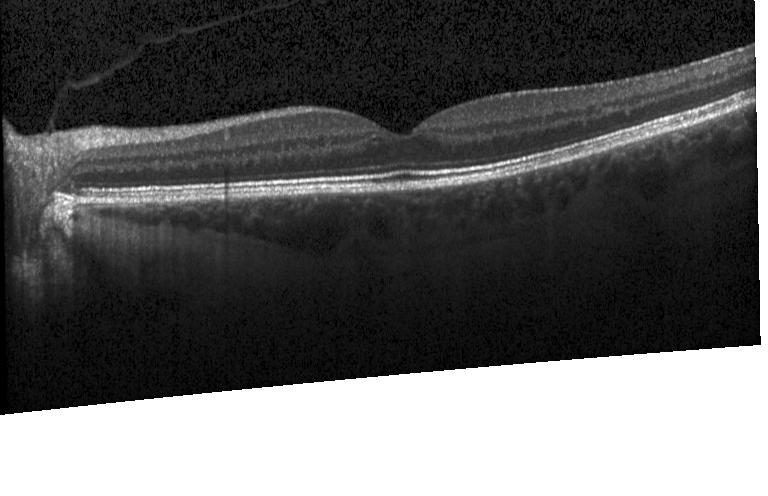

OCT line scan · spectral-domain OCT · acquired on a Heidelberg Spectralis.
This B-scan demonstrates no CNV, DME, or drusen.